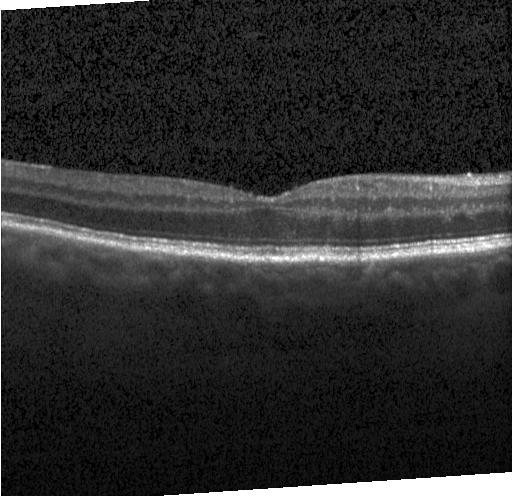 Macular scan · OCT B-scan — Dx: neither CNV, DME, nor drusen.